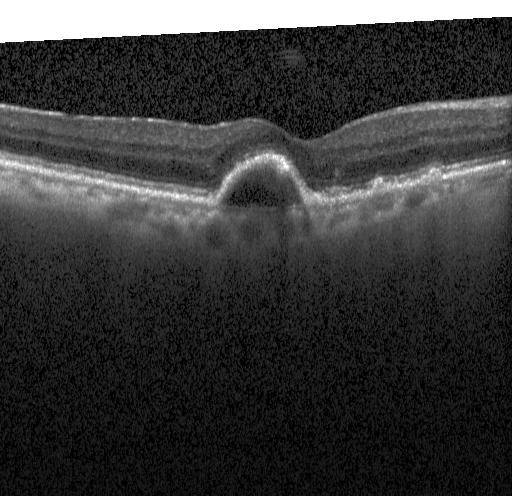
Heidelberg Spectralis OCT system, retinal OCT cross-section.
Diagnosis: CNV.